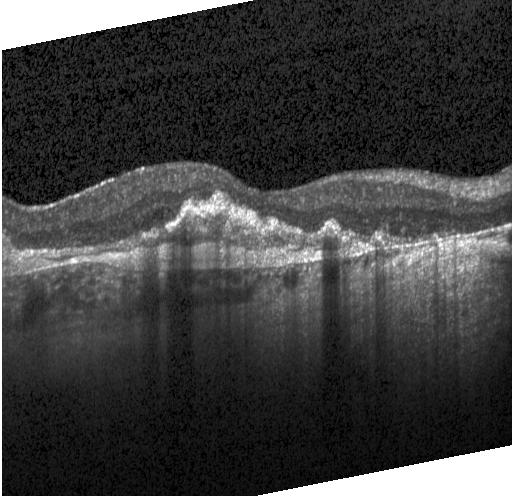
Centered on the fovea · instrument: Heidelberg Spectralis · spectral-domain OCT · optical coherence tomography B-scan — Finding: choroidal neovascularization (CNV).